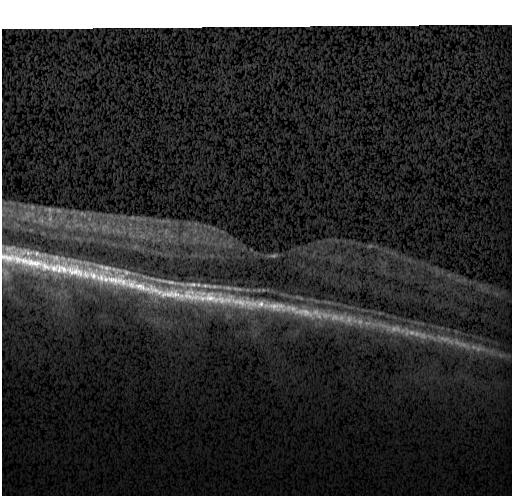 Retinal OCT cross-section. Heidelberg Spectralis OCT system.
Diagnosis: no choroidal neovascularization, no diabetic macular edema, and no drusen.